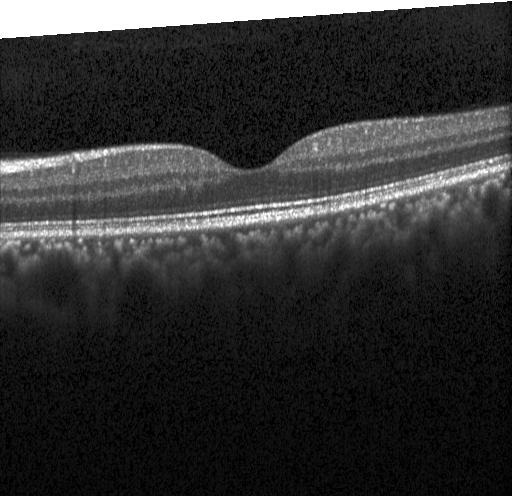 Retinal OCT cross-section, acquired on a Heidelberg Spectralis, centered on the fovea
Finding: no CNV, DME, or drusen.